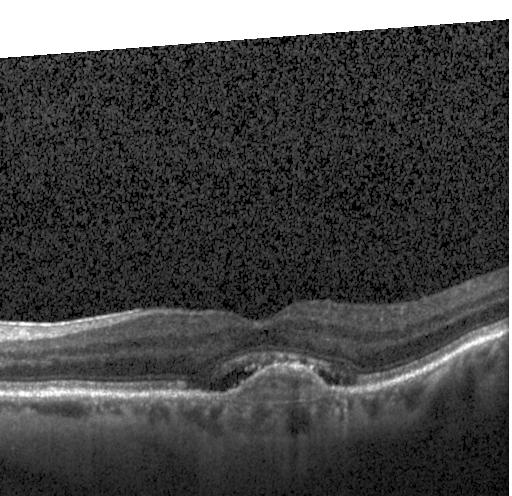
Spectral-domain optical coherence tomography. Instrument: Heidelberg Spectralis. Horizontal scan through the fovea. Optical coherence tomography B-scan. Finding: choroidal neovascularization (CNV).